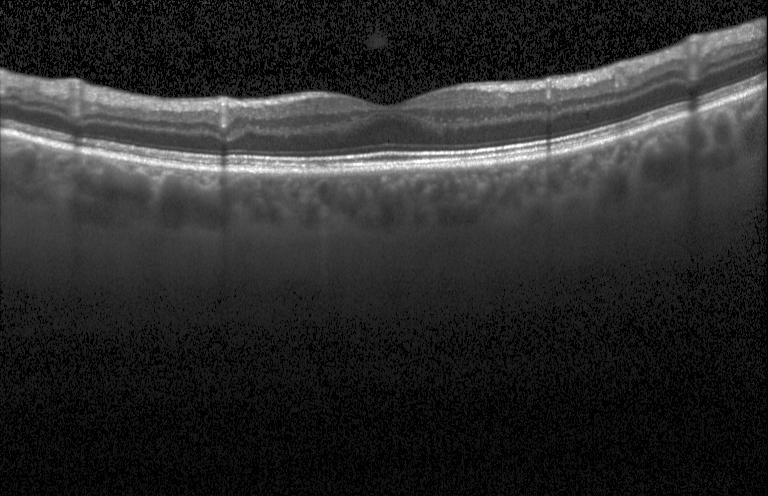 Retinal OCT cross-section; through the macula; spectral-domain OCT — This B-scan demonstrates neither CNV, DME, nor drusen.